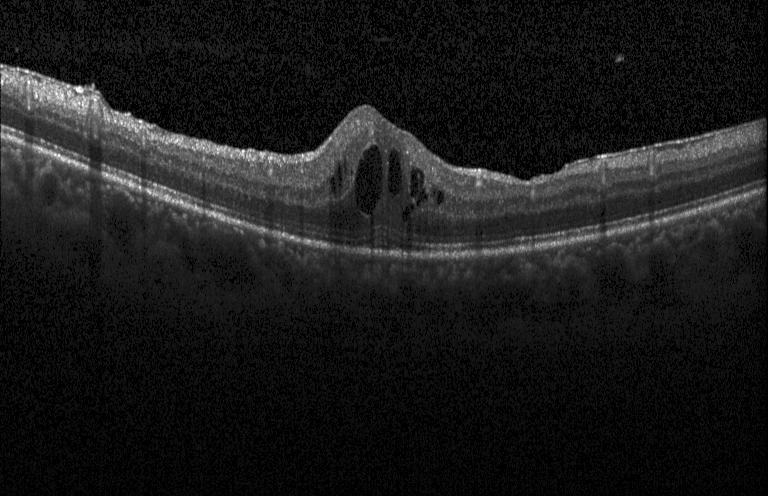
OCT finding: diabetic macular edema.